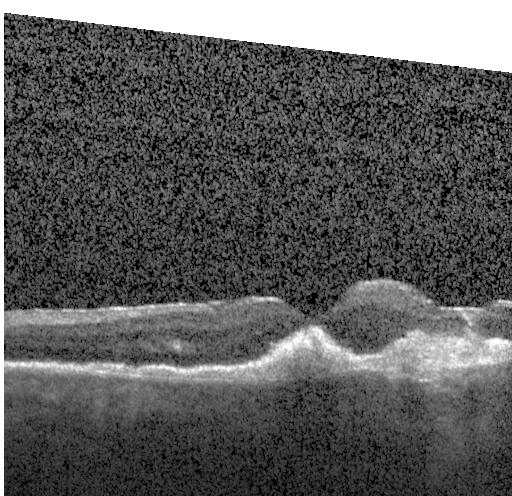 Instrument: Heidelberg Spectralis · OCT line scan
Assessment: CNV.